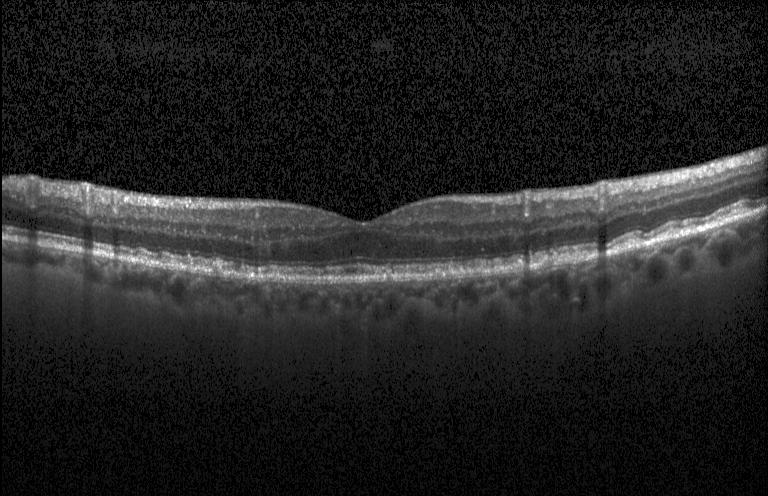
OCT scan showing multiple drusen.